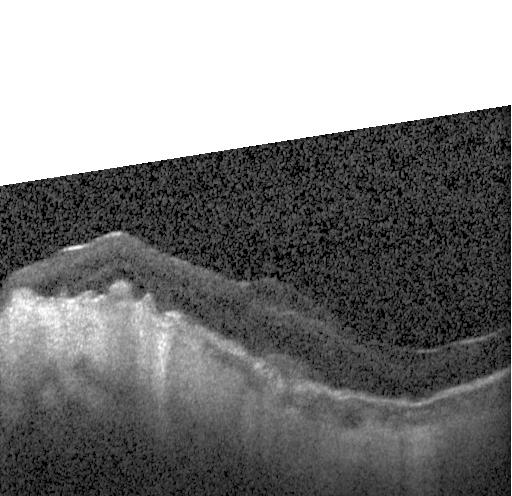
OCT B-scan showing choroidal neovascularization (CNV).